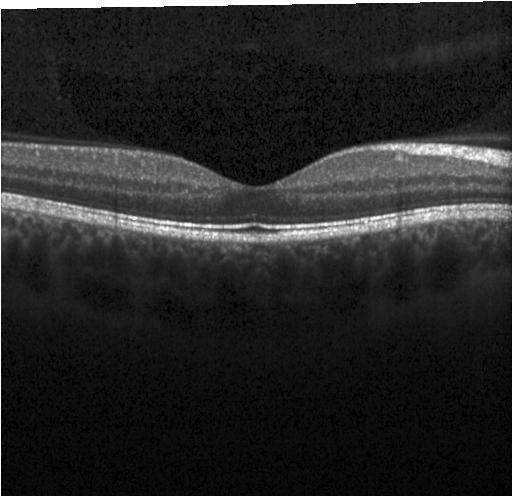
Horizontal scan through the fovea, spectral-domain OCT, acquired on a Heidelberg Spectralis, OCT B-scan. OCT finding: no choroidal neovascularization, diabetic macular edema, or drusen.